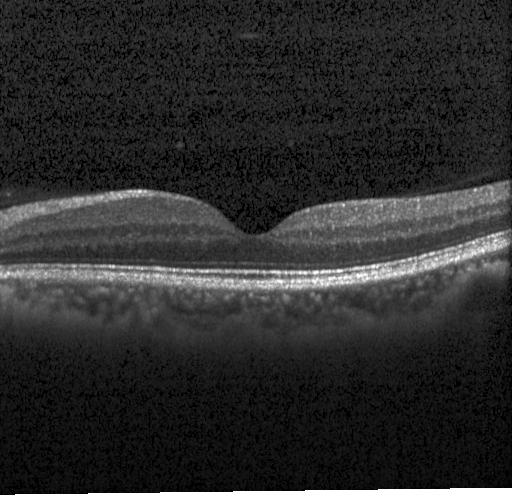
Spectral-domain optical coherence tomography. Heidelberg Spectralis. Retinal OCT B-scan. Impression: no evidence of choroidal neovascularization, diabetic macular edema, or drusen.